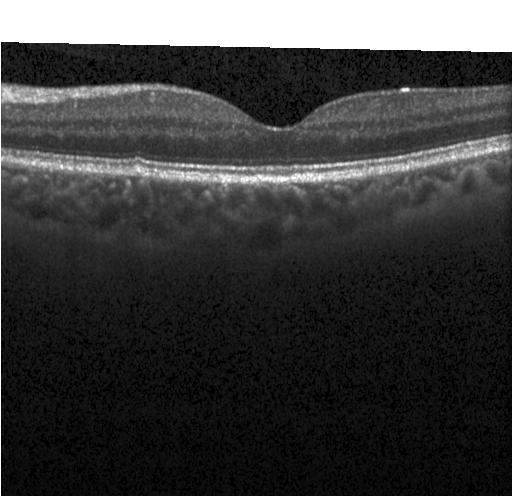 Retinal OCT B-scan · acquired on a Heidelberg Spectralis · horizontal scan through the fovea
OCT finding: drusen.